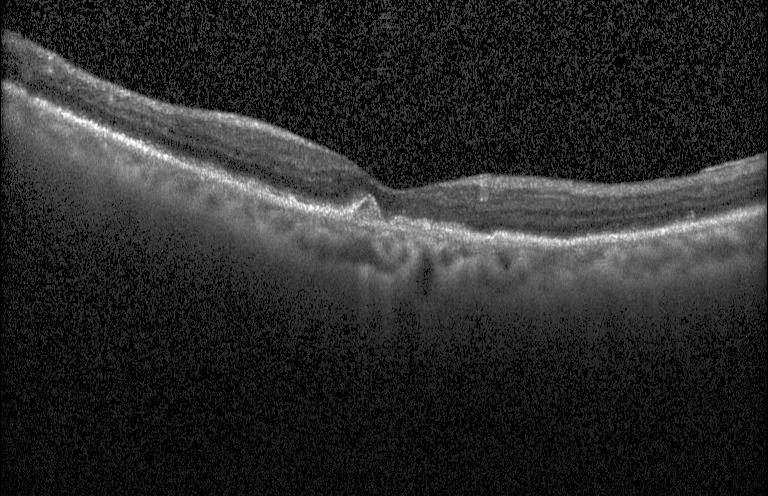

Retinal OCT B-scan.
Assessment: choroidal neovascularization.